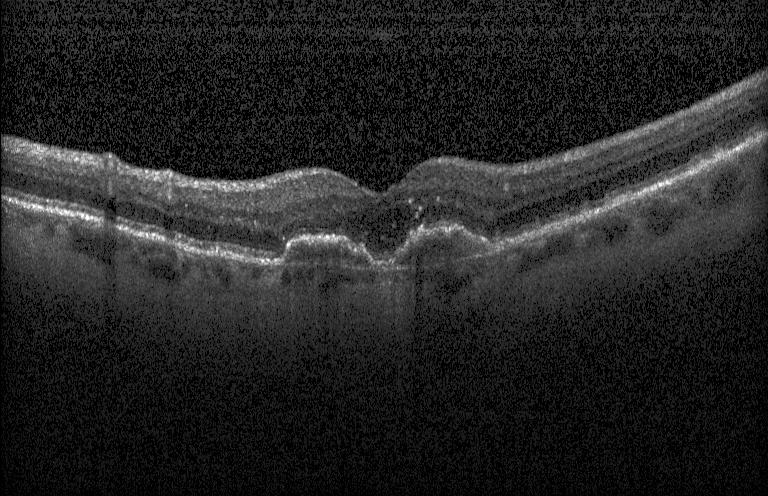 OCT finding: choroidal neovascularization.